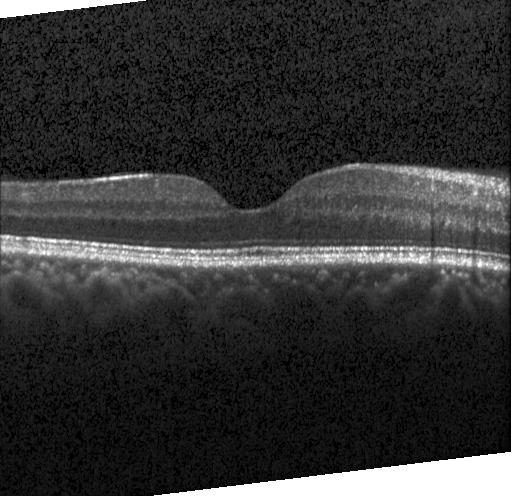
OCT B-scan. Impression: no evidence of choroidal neovascularization, diabetic macular edema, or drusen.